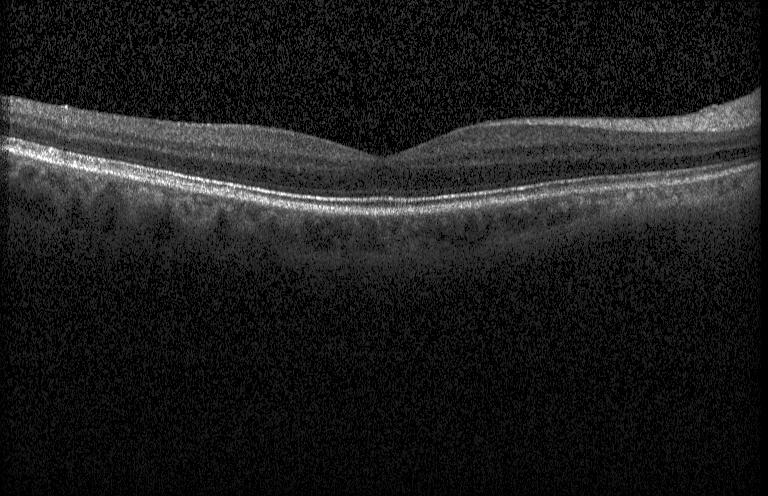
No choroidal neovascularization, no diabetic macular edema, and no drusen.